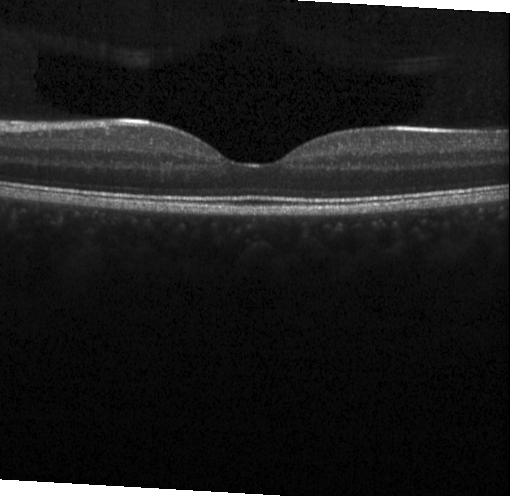
Fovea-centered · spectral-domain optical coherence tomography · Heidelberg Spectralis · OCT B-scan.
This B-scan demonstrates no evidence of CNV, DME, or drusen.